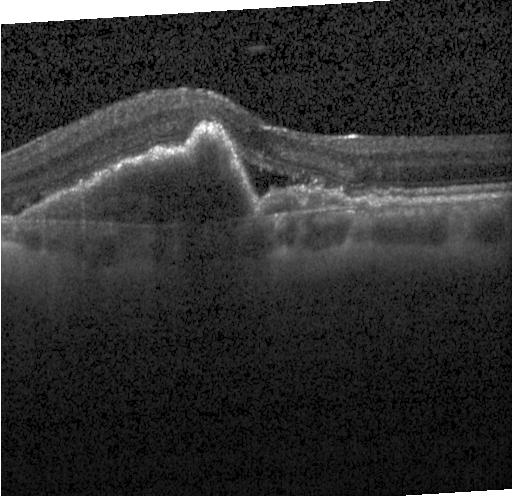

Heidelberg Spectralis OCT system, through the macula, spectral-domain optical coherence tomography, optical coherence tomography scan
Assessment: a choroidal neovascular membrane.